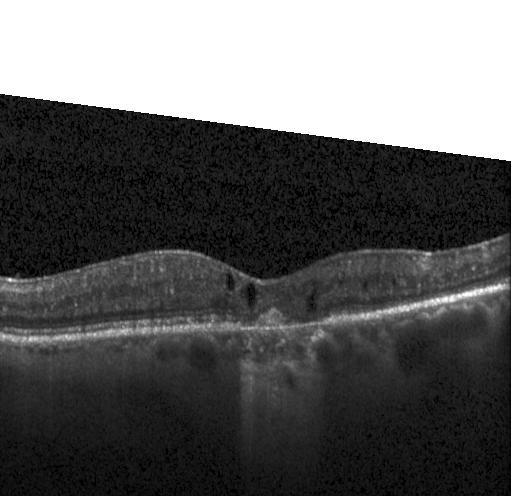 Optical coherence tomography B-scan — Impression: a choroidal neovascular membrane.